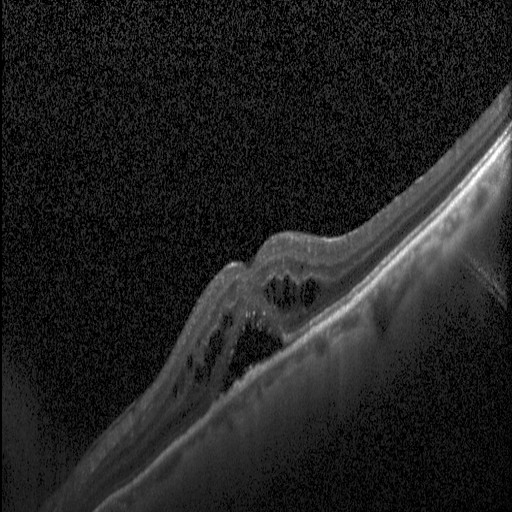
Macular OCT demonstrating diabetic macular edema (DME).